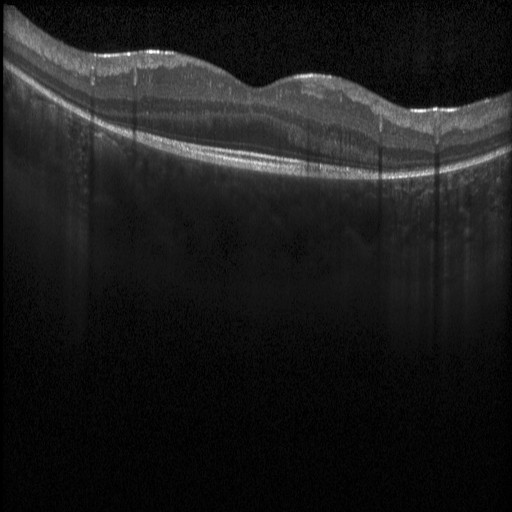 Optical coherence tomography scan · centered on the fovea.
Diagnosis: diabetic macular edema.